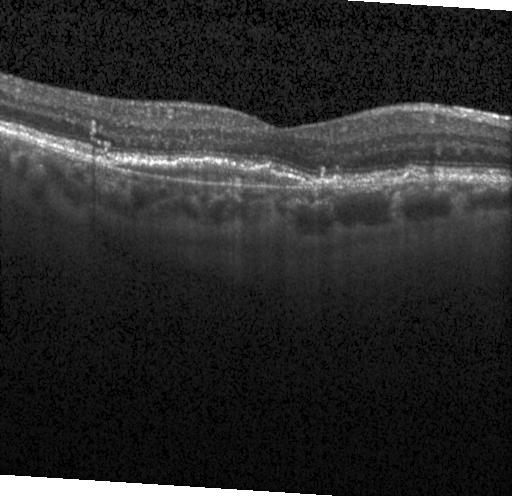 Macular OCT demonstrating CNV.